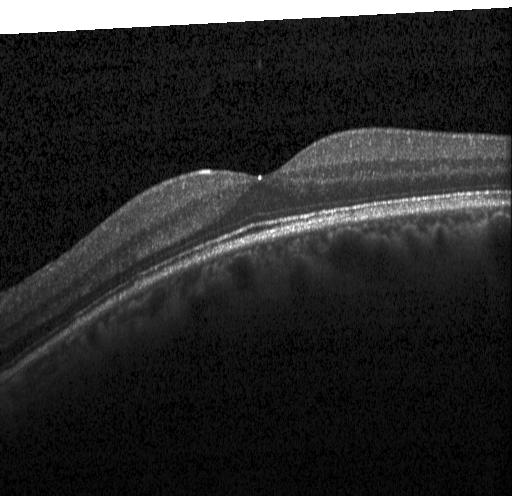

OCT B-scan
Finding: no evidence of choroidal neovascularization, diabetic macular edema, or drusen.